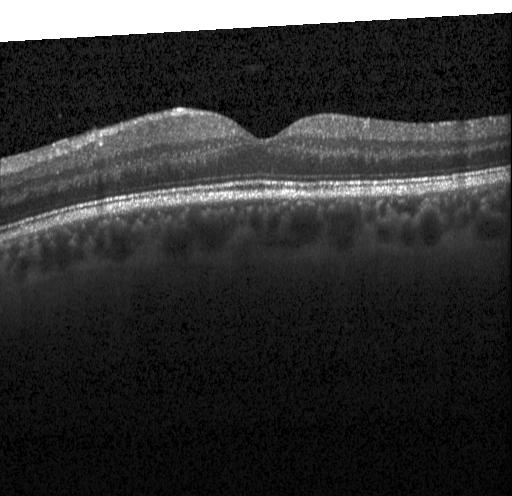

OCT B-scan
OCT finding: no evidence of choroidal neovascularization, diabetic macular edema, or drusen.